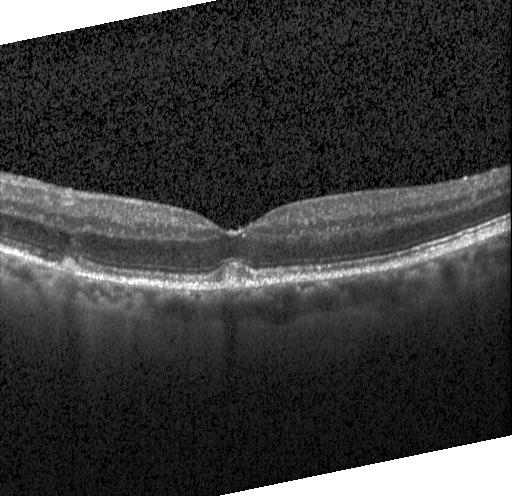 Dx: drusen.